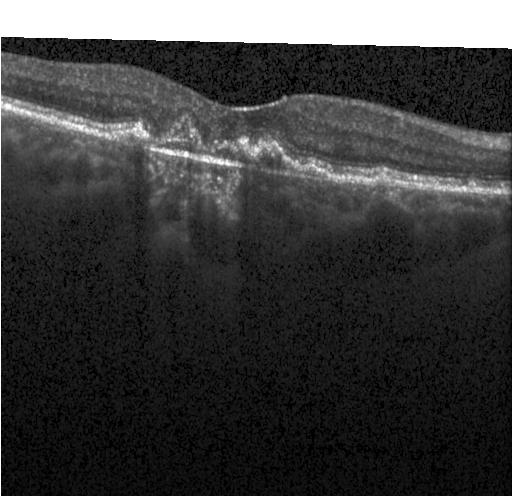

Dx: choroidal neovascularization (CNV).